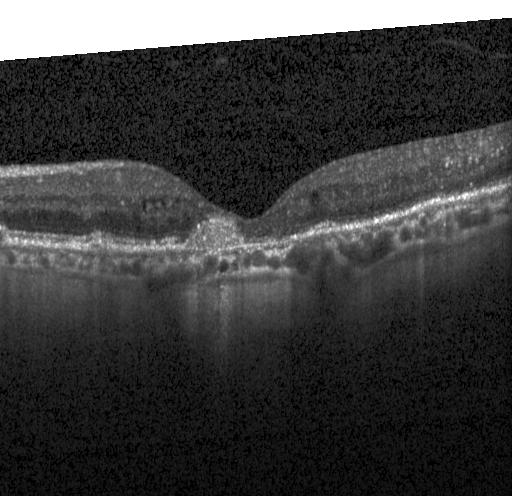 Diagnosis: choroidal neovascularization (CNV).